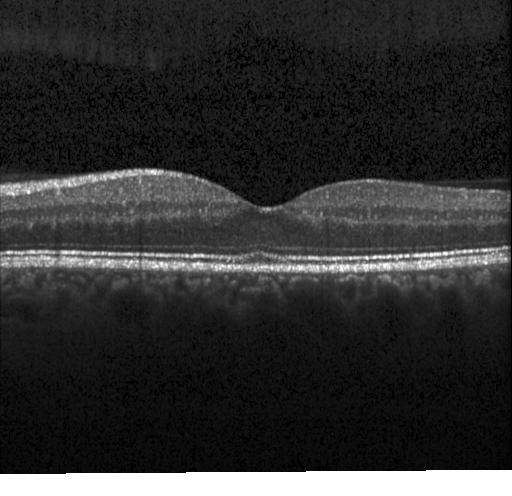

Finding: no evidence of choroidal neovascularization, diabetic macular edema, or drusen.